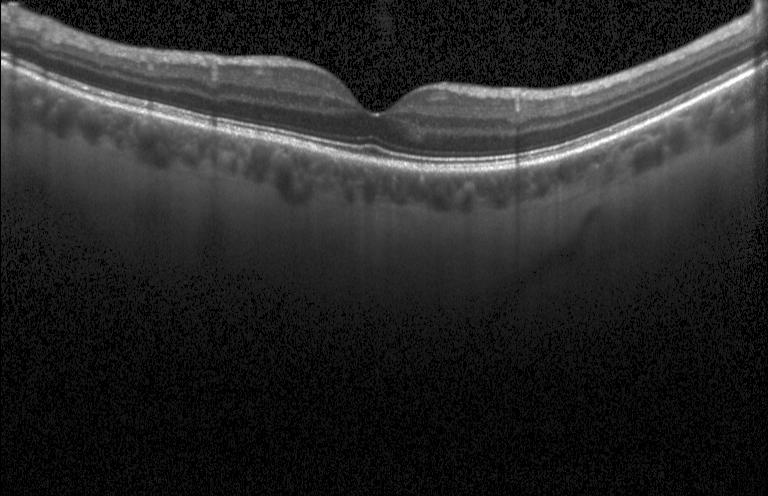 Optical coherence tomography scan. Macular scan.
Assessment: neither choroidal neovascularization, diabetic macular edema, nor drusen.